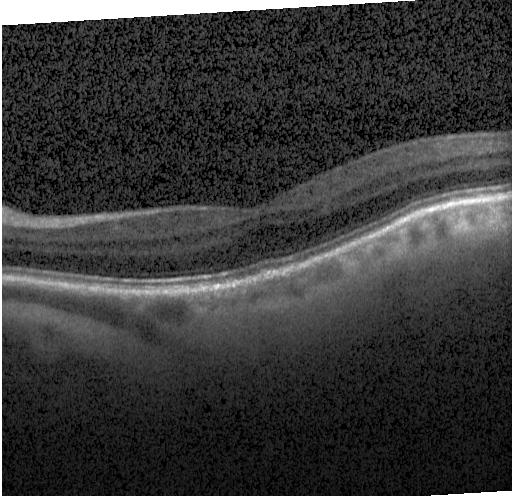 Retinal OCT B-scan · spectral-domain OCT. OCT finding: neither choroidal neovascularization, diabetic macular edema, nor drusen.